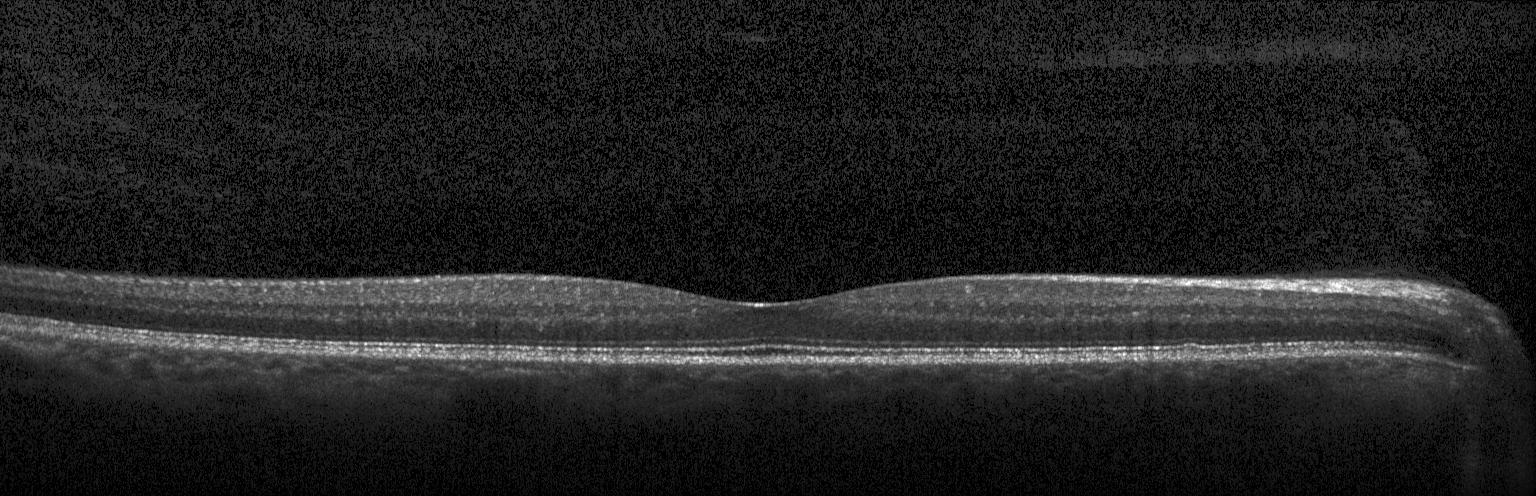

Retinal OCT B-scan — No evidence of choroidal neovascularization, diabetic macular edema, or drusen.